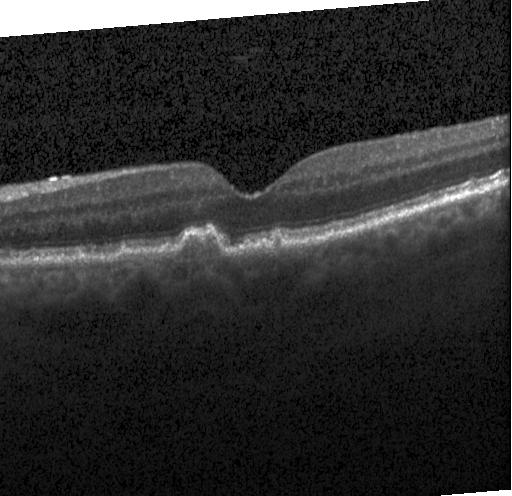

Centered on the fovea · retinal OCT cross-section · Heidelberg Spectralis.
Impression: drusen.